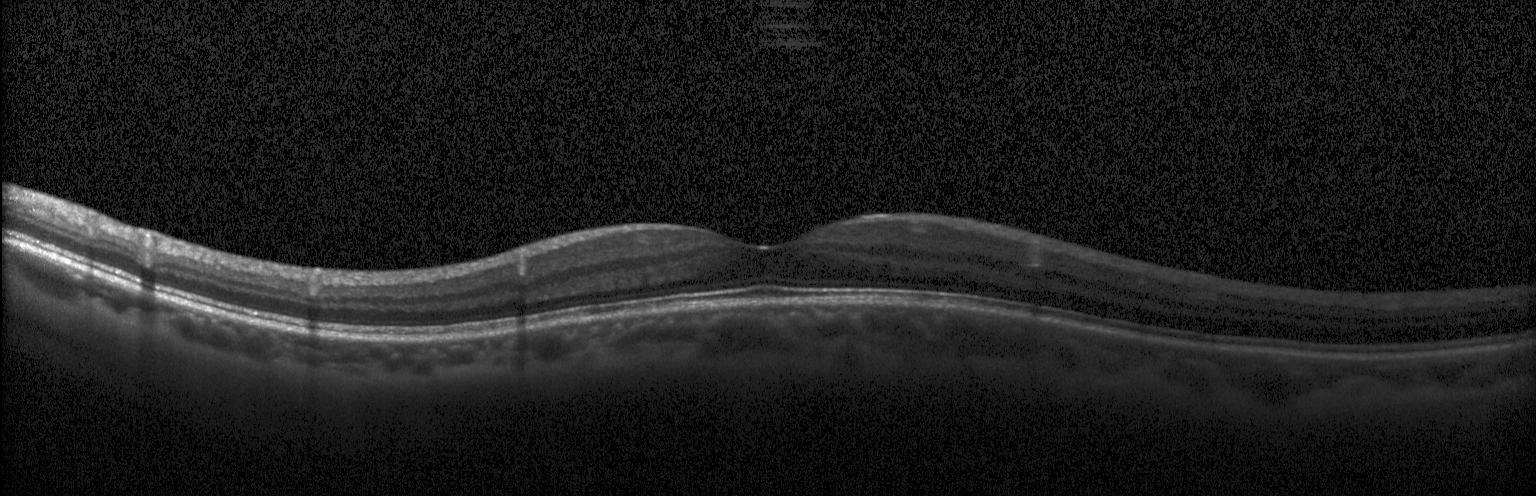
No choroidal neovascularization, no diabetic macular edema, and no drusen.